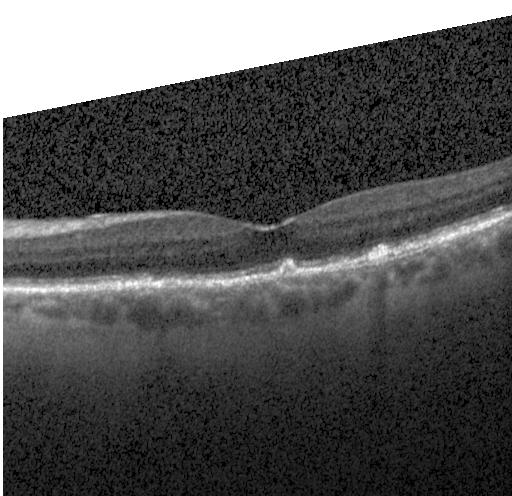
Spectral-domain optical coherence tomography. Retinal OCT cross-section — Finding: drusen.